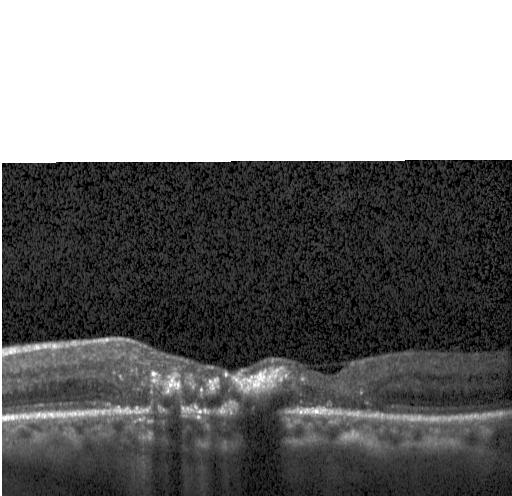 OCT B-scan, through the macula, spectral-domain optical coherence tomography
CNV.